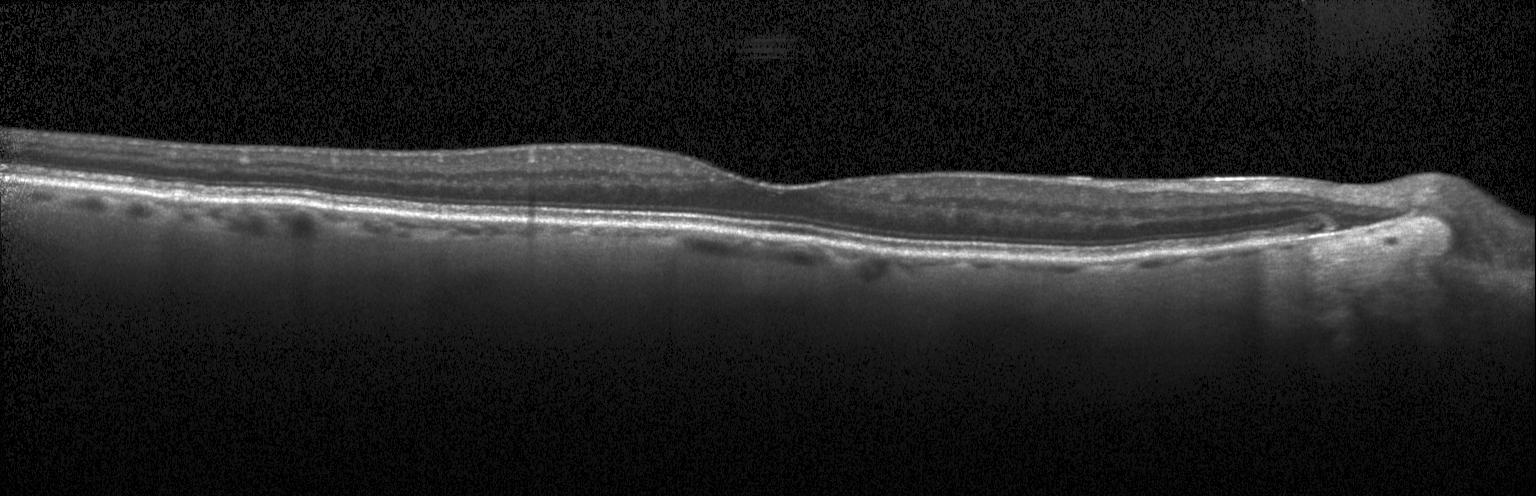
OCT line scan
This B-scan demonstrates no evidence of choroidal neovascularization, diabetic macular edema, or drusen.